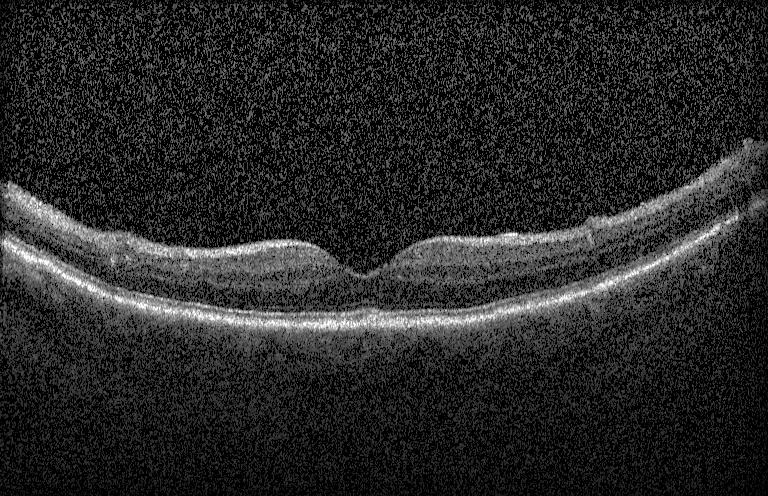

Centered on the fovea. OCT line scan. Spectral-domain optical coherence tomography. Instrument: Heidelberg Spectralis
The scan shows no CNV, DME, or drusen.